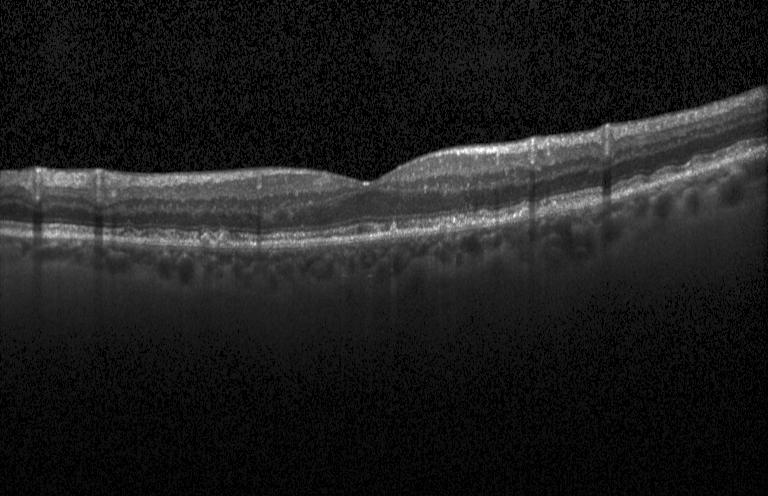 Heidelberg Spectralis OCT system, OCT B-scan, macular scan — Impression: multiple drusen.